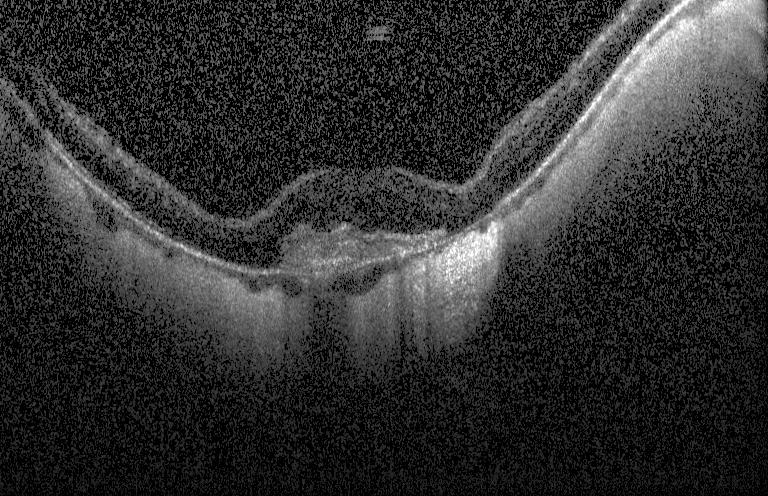 OCT B-scan showing CNV.